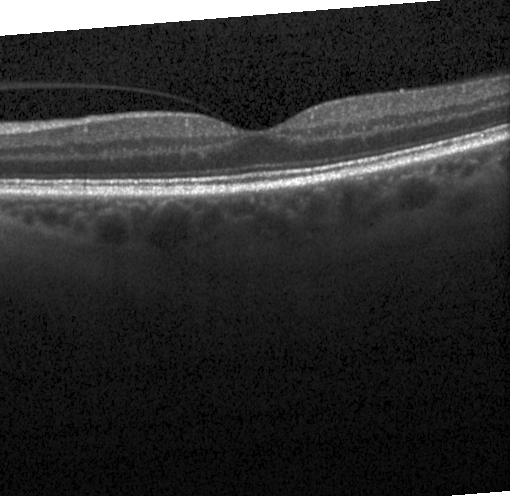 SD-OCT. Centered on the fovea. Optical coherence tomography B-scan. Acquired on a Heidelberg Spectralis. Dx: no choroidal neovascularization, no diabetic macular edema, and no drusen.